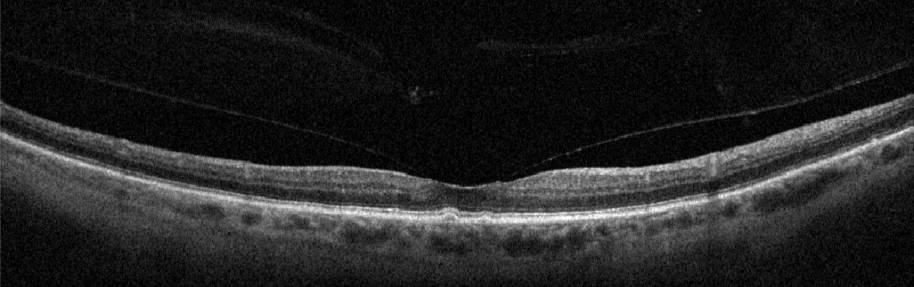 Dx: age-related macular degeneration (AMD).